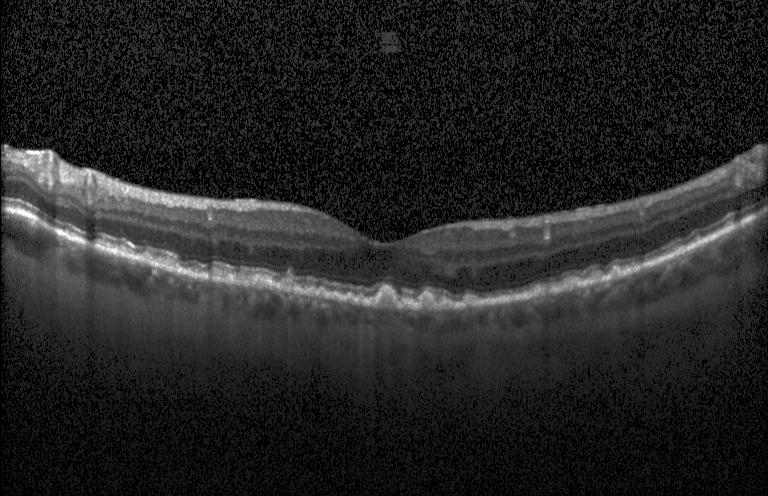

OCT line scan — Sub-RPE drusenoid deposits.